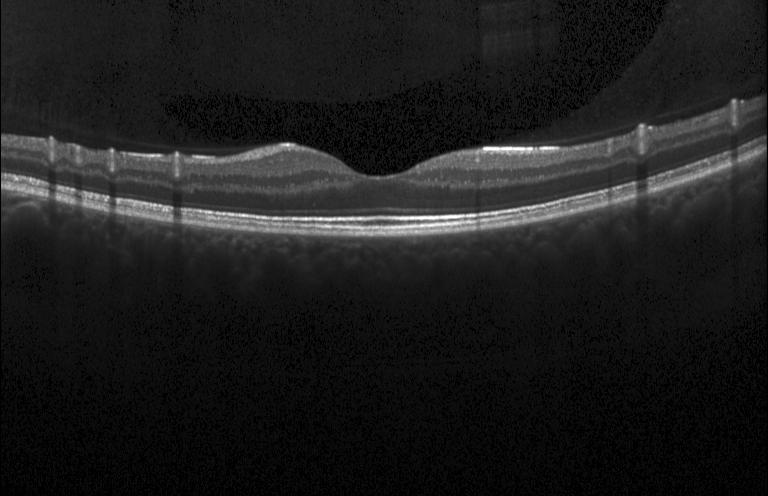
OCT B-scan showing no evidence of choroidal neovascularization, diabetic macular edema, or drusen.